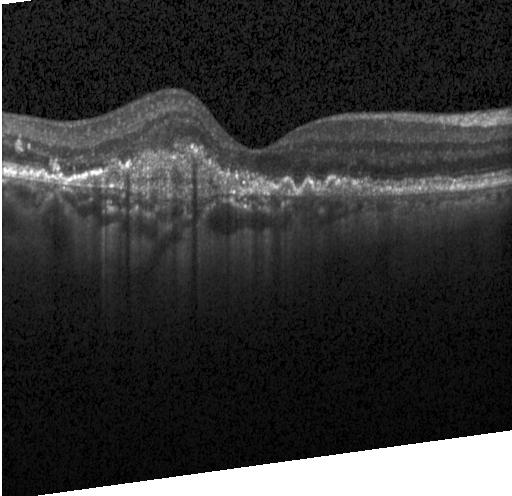
Retinal OCT cross-section.
Finding: a choroidal neovascular membrane.